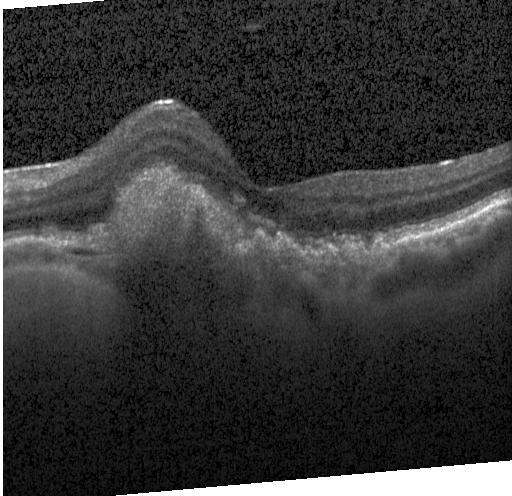 Retinal OCT B-scan. This B-scan demonstrates a choroidal neovascular membrane.